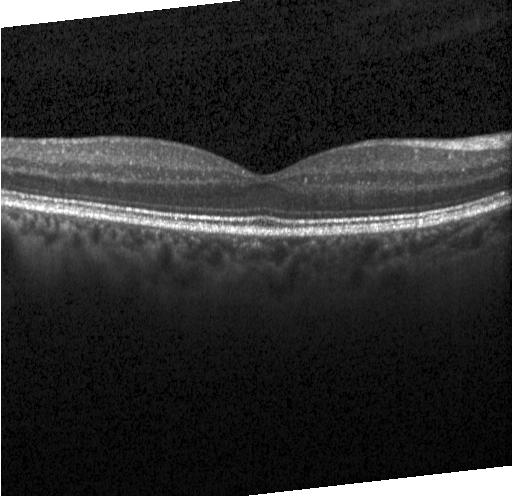 Optical coherence tomography B-scan.
Finding: no choroidal neovascularization, diabetic macular edema, or drusen.